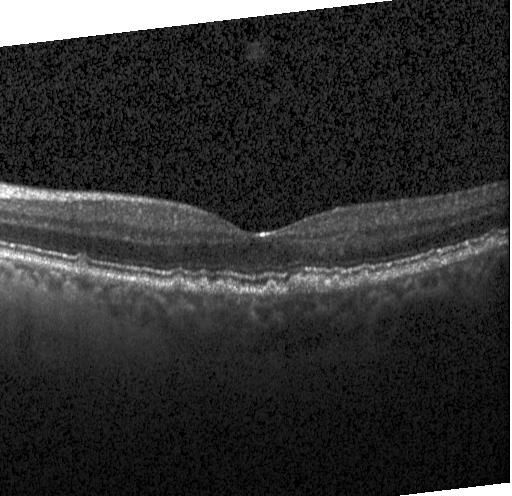 Instrument: Heidelberg Spectralis · OCT line scan · spectral-domain optical coherence tomography · fovea-centered.
Multiple drusen.